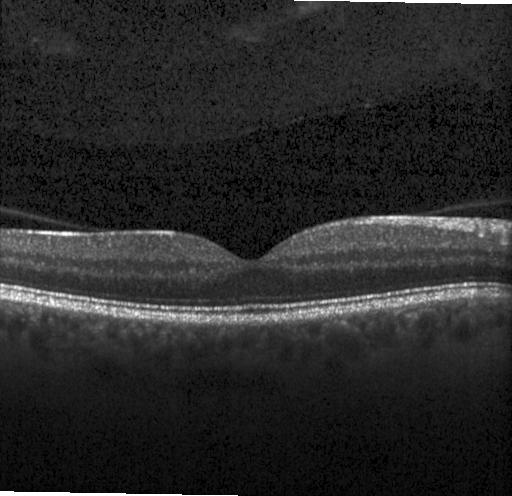

OCT scan showing no CNV, DME, or drusen.